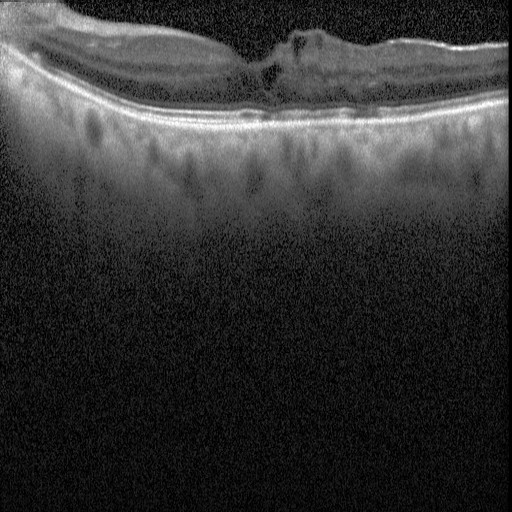

Fovea-centered · OCT B-scan. Dx: DME.